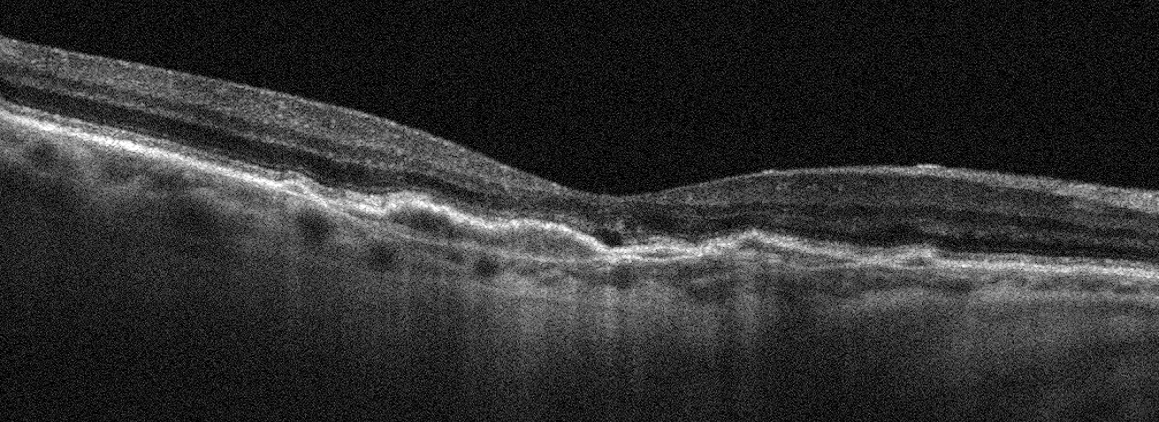

Optical coherence tomography scan, oculus dexter.
This B-scan demonstrates AMD.